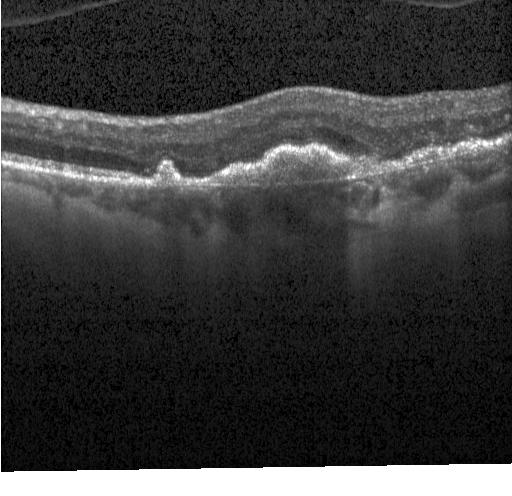 Through the macula · OCT line scan · instrument: Heidelberg Spectralis — Impression: a choroidal neovascular membrane.